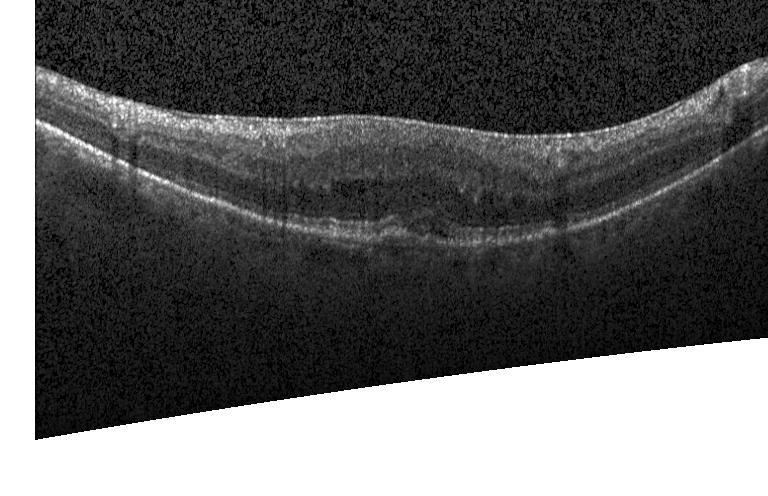

Assessment: a choroidal neovascular membrane.